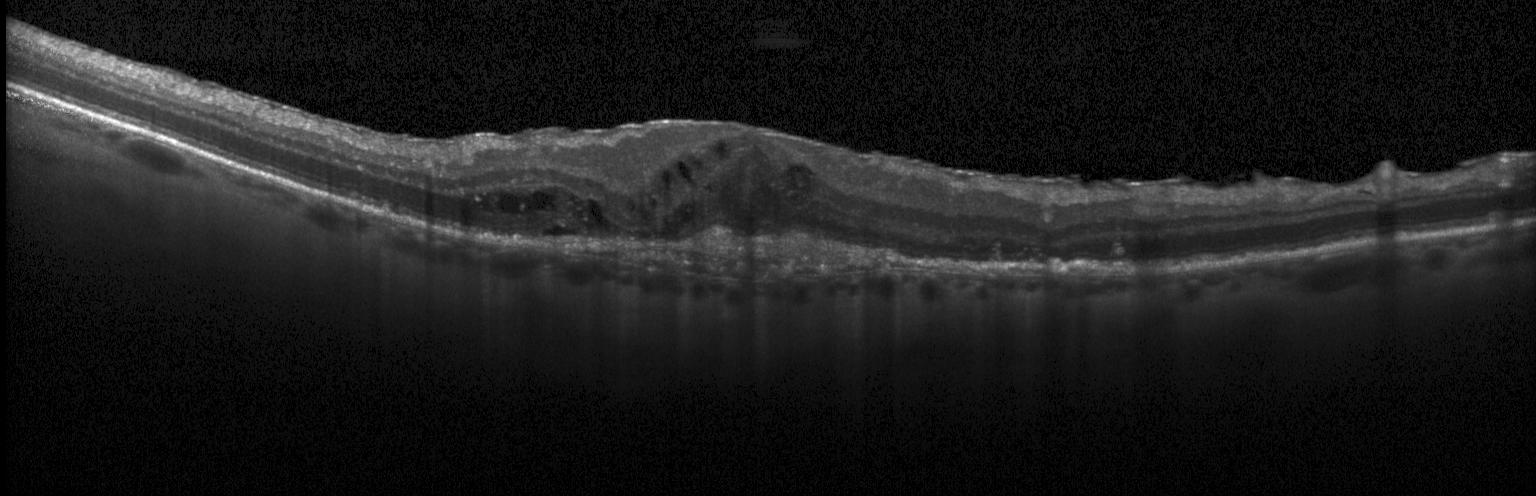 Finding: CNV.